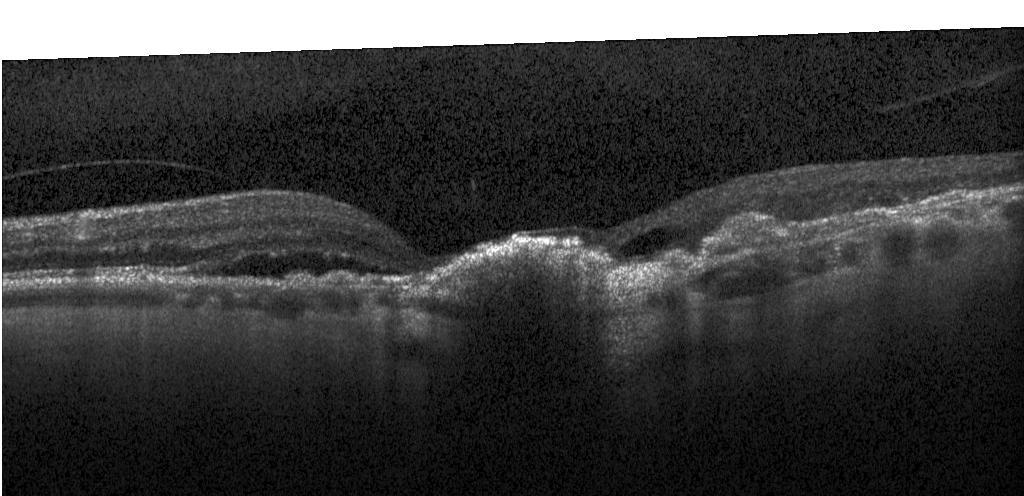
Retinal OCT B-scan. Spectral-domain OCT
Macular OCT: a choroidal neovascular membrane.